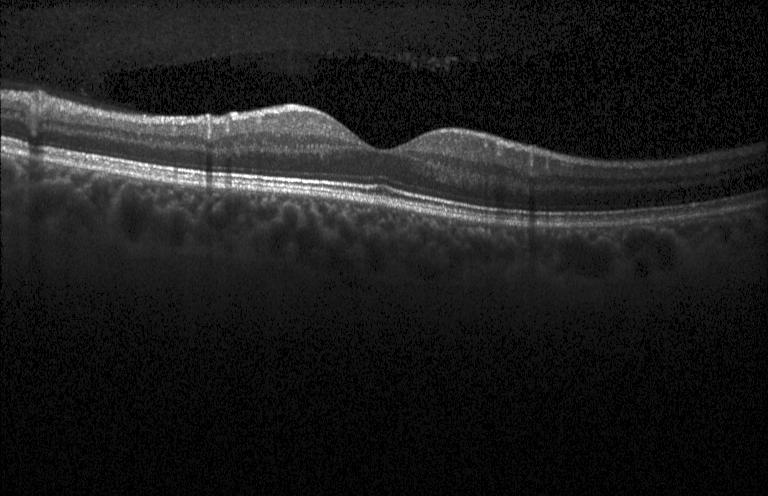 Optical coherence tomography scan; spectral-domain OCT; acquired on a Heidelberg Spectralis; macular scan — This B-scan demonstrates no evidence of CNV, DME, or drusen.